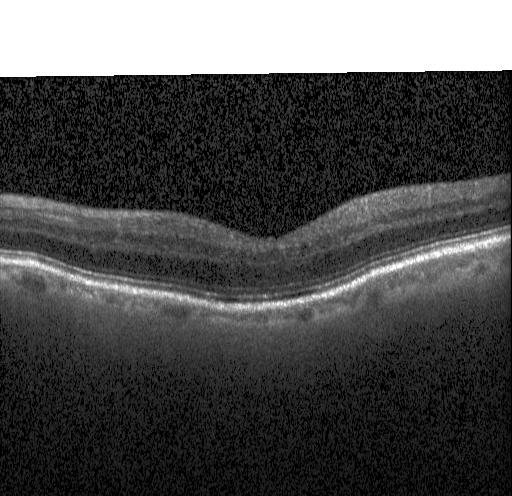

Retinal OCT cross-section, horizontal scan through the fovea — This B-scan demonstrates neither choroidal neovascularization, diabetic macular edema, nor drusen.